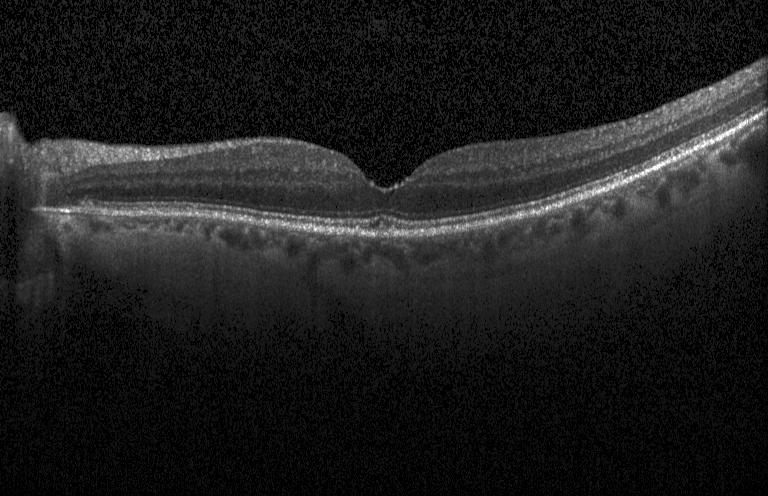
Diagnosis: neither choroidal neovascularization, diabetic macular edema, nor drusen.